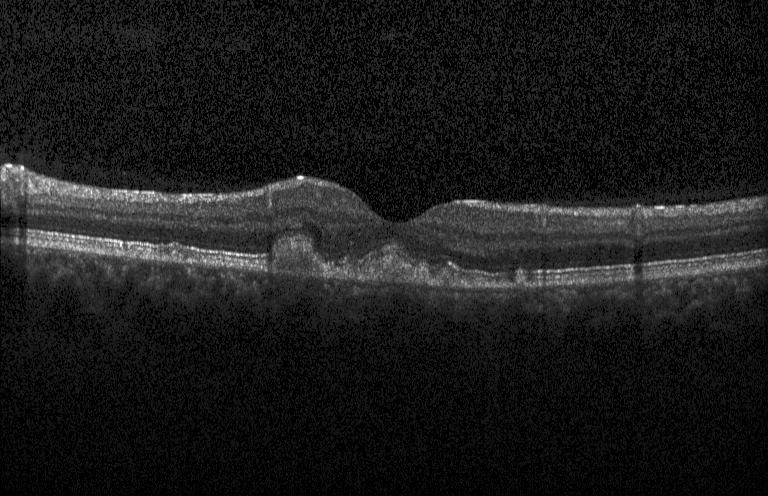 Retinal OCT cross-section; centered on the fovea; acquired on a Heidelberg Spectralis — The scan shows sub-RPE drusenoid deposits.